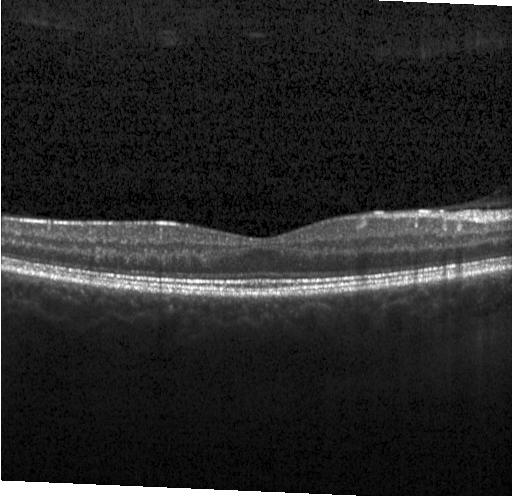
SD-OCT, horizontal scan through the fovea, OCT B-scan. Diagnosis: no choroidal neovascularization, diabetic macular edema, or drusen.